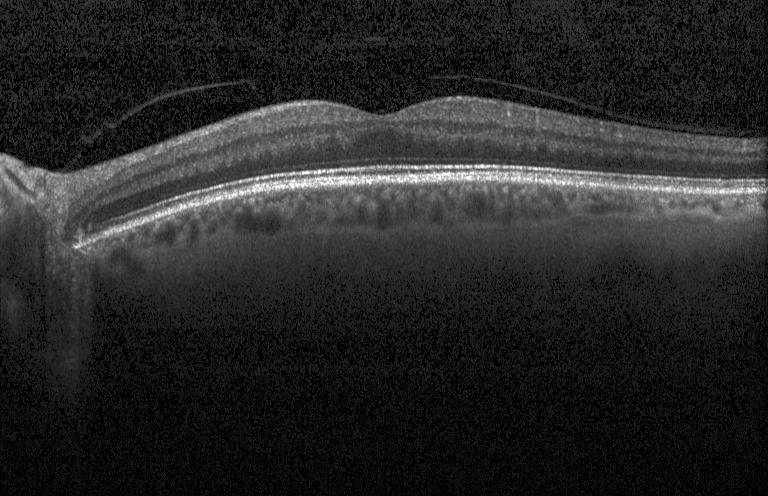

Retinal OCT cross-section — The scan shows no choroidal neovascularization, no diabetic macular edema, and no drusen.